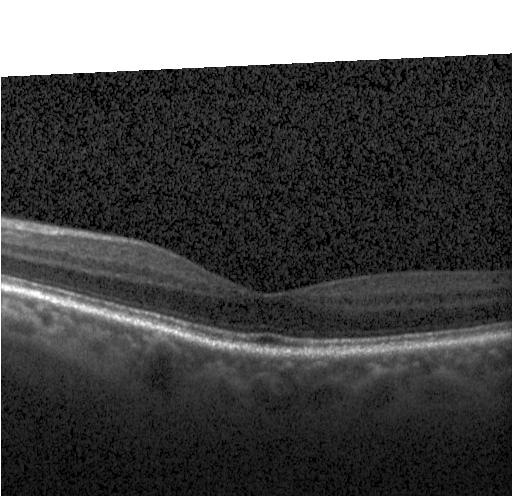

OCT B-scan · horizontal scan through the fovea. This B-scan demonstrates neither choroidal neovascularization, diabetic macular edema, nor drusen.